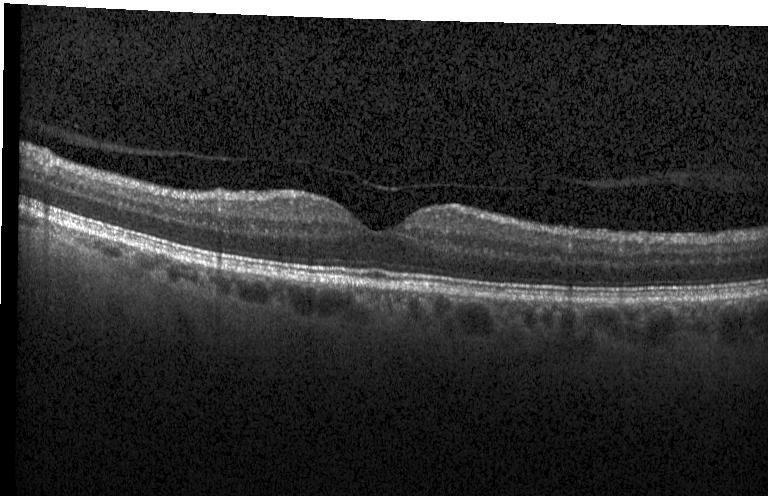

Spectral-domain OCT B-scan: neither CNV, DME, nor drusen.